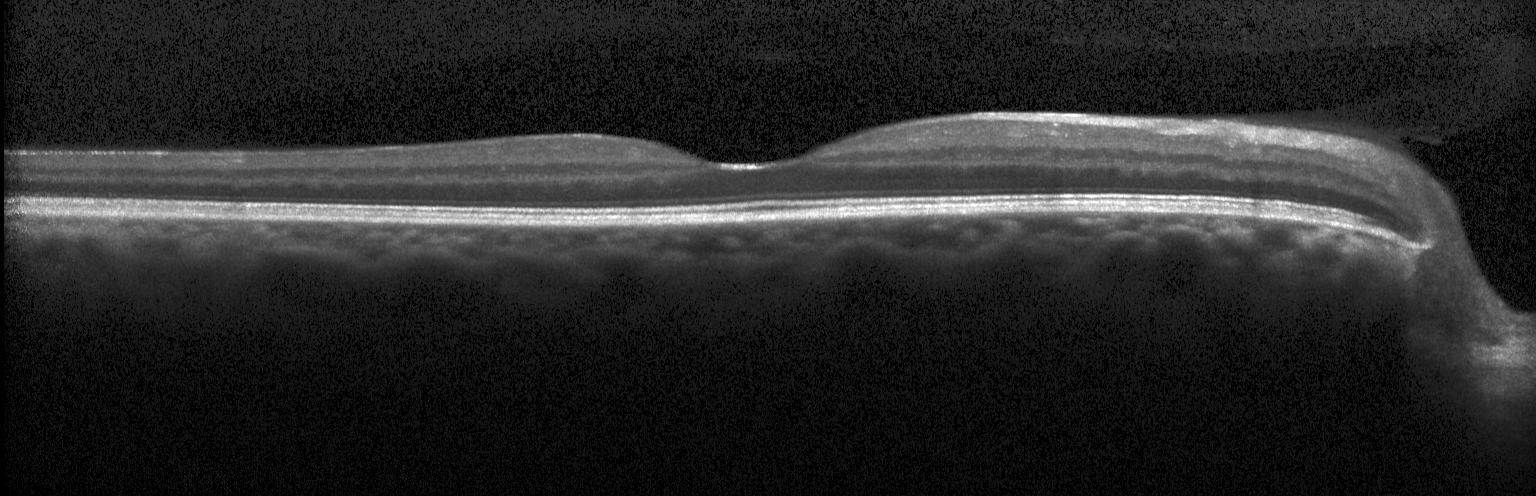 Heidelberg Spectralis; OCT B-scan; spectral-domain optical coherence tomography; horizontal scan through the fovea — Finding: no choroidal neovascularization, diabetic macular edema, or drusen.